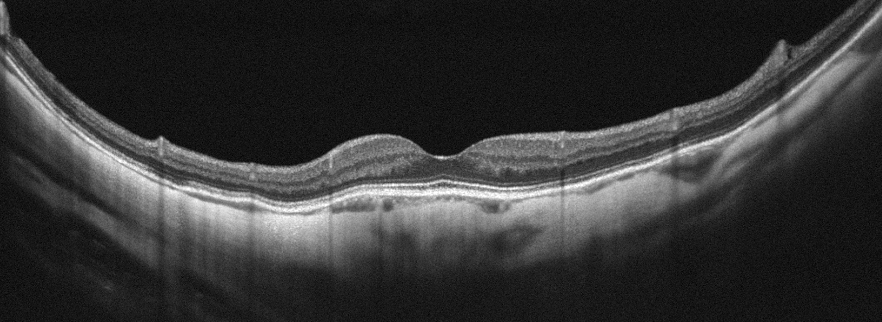
Instrument: Optovue Avanti RTVue XR; oculus sinister; retinal OCT cross-section — Impression: no AMD, DME, ERM, RAO, RVO, or VID.